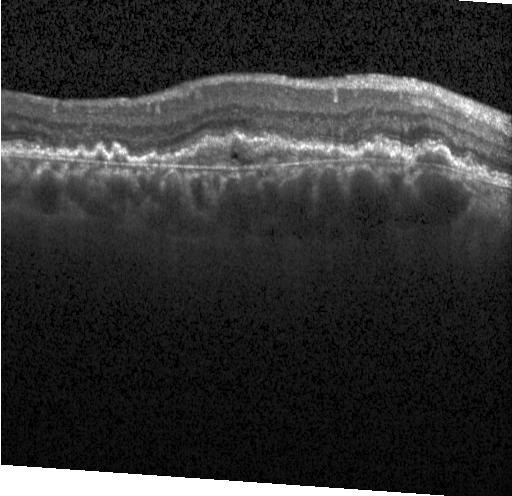 Assessment: choroidal neovascularization.